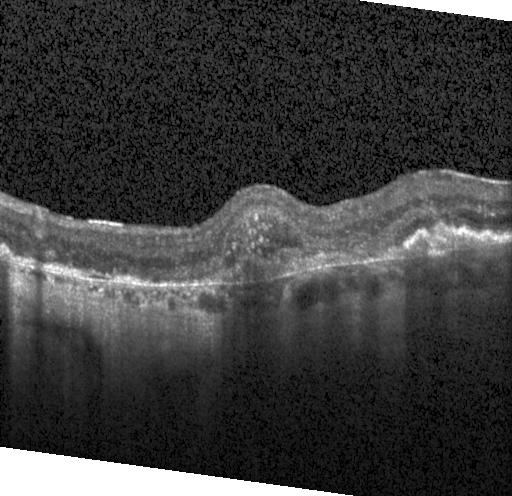 Centered on the fovea, OCT B-scan.
Finding: choroidal neovascularization (CNV).